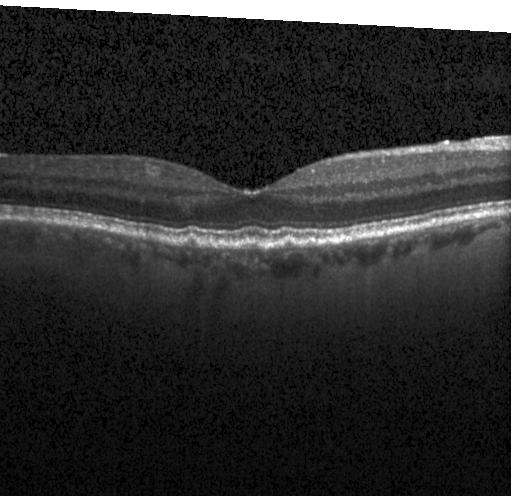
Optical coherence tomography scan — Finding: drusen.